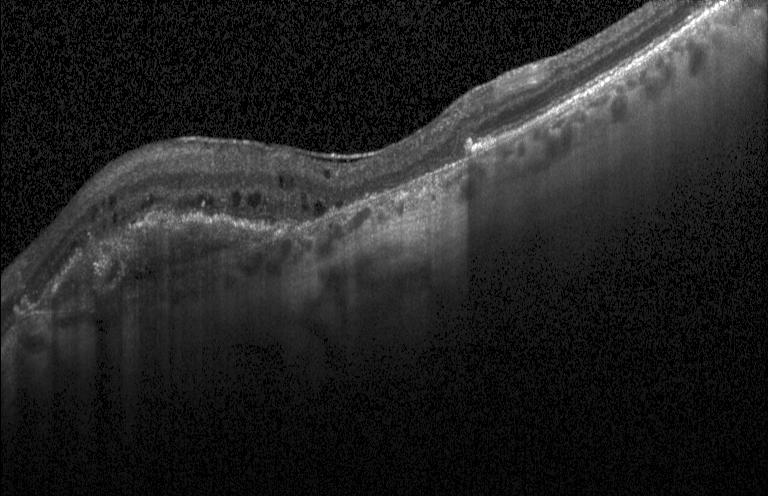 Retinal OCT B-scan; Heidelberg Spectralis OCT system
Dx: a choroidal neovascular membrane.